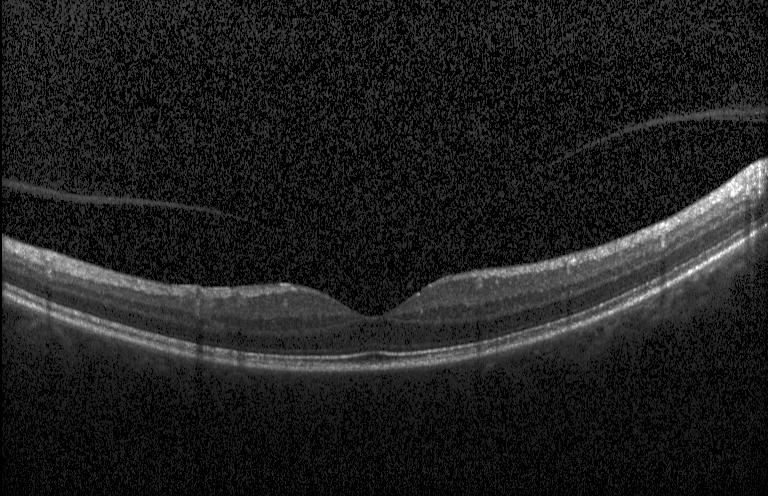

OCT scan showing neither choroidal neovascularization, diabetic macular edema, nor drusen.